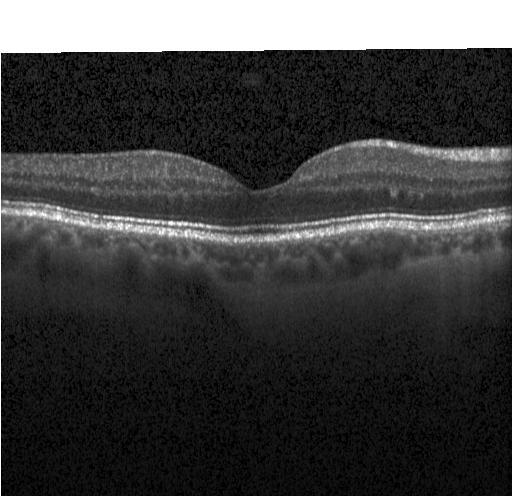 OCT scan showing neither choroidal neovascularization, diabetic macular edema, nor drusen.